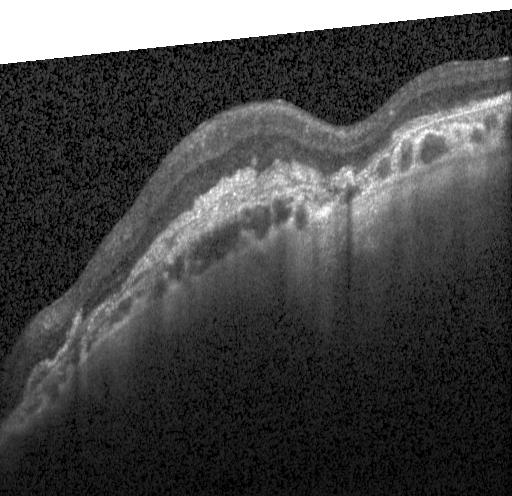 Spectral-domain optical coherence tomography, retinal OCT cross-section. Finding: CNV.